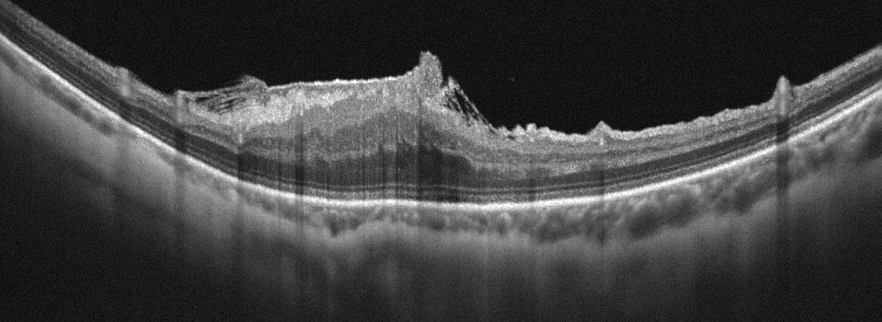

Left eye · optical coherence tomography scan — This B-scan demonstrates ERM.